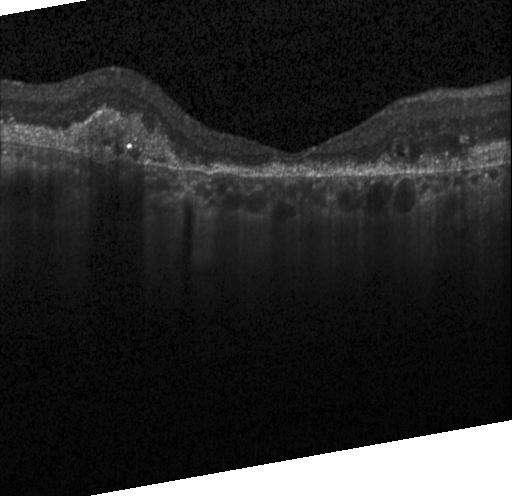
OCT B-scan · through the macula · spectral-domain optical coherence tomography — Finding: choroidal neovascularization (CNV).